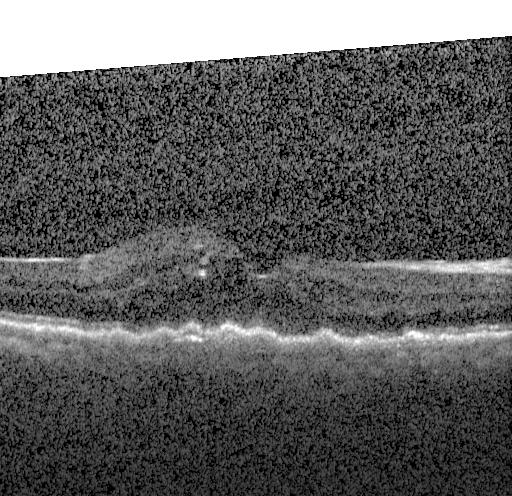

Macular scan; SD-OCT; OCT line scan; instrument: Heidelberg Spectralis.
Impression: choroidal neovascularization (CNV).